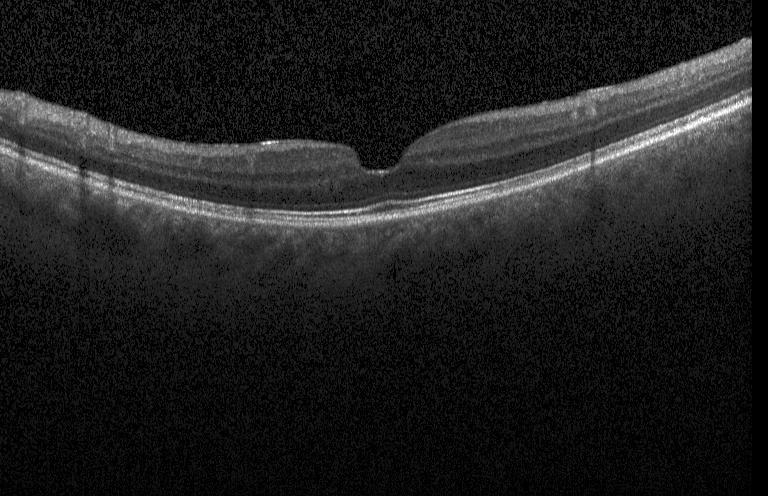

OCT B-scan showing neither choroidal neovascularization, diabetic macular edema, nor drusen.